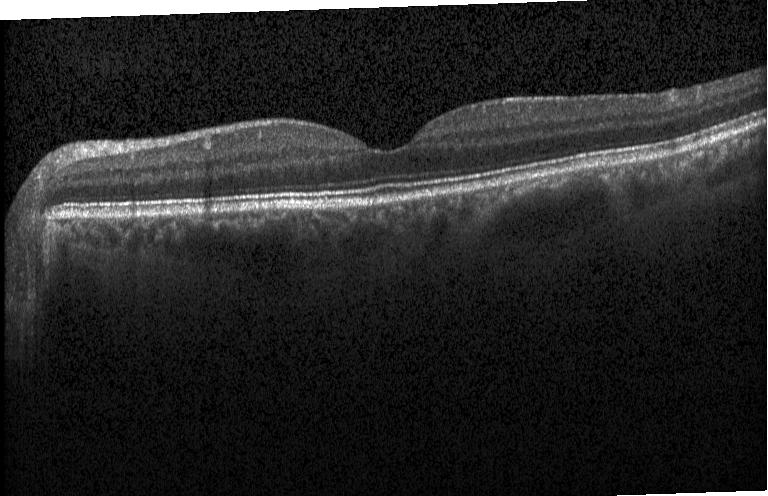 OCT B-scan.
No evidence of choroidal neovascularization, diabetic macular edema, or drusen.